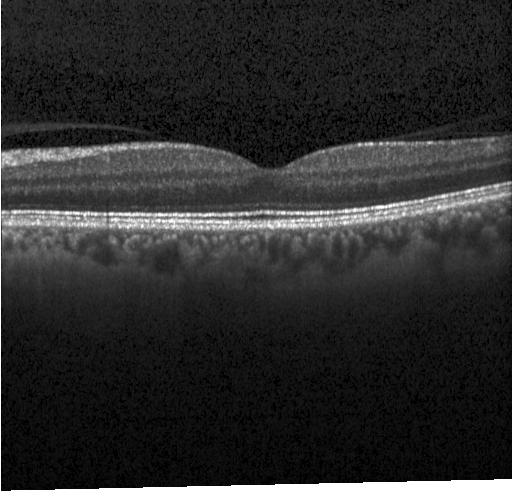 OCT B-scan showing no choroidal neovascularization, no diabetic macular edema, and no drusen.